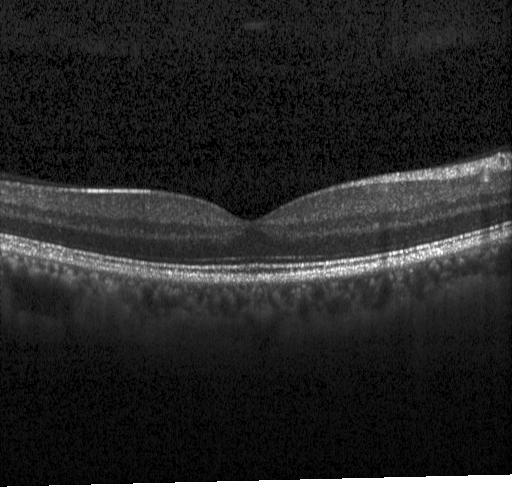
Spectral-domain OCT B-scan: no choroidal neovascularization, diabetic macular edema, or drusen.